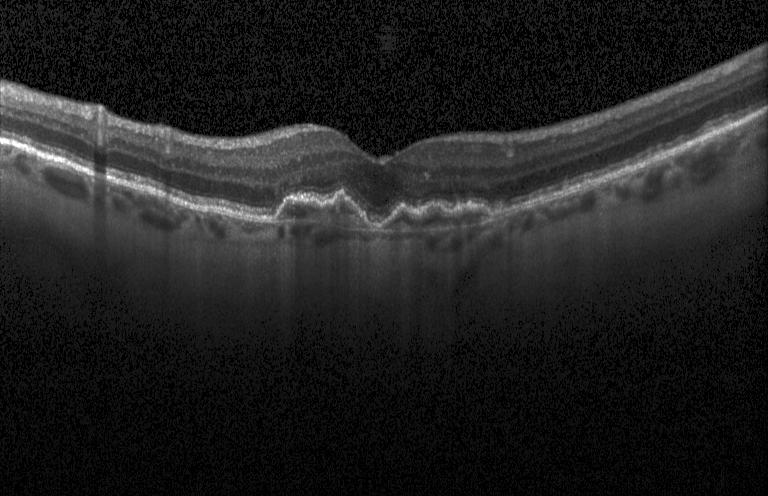 Macular scan. Optical coherence tomography scan. SD-OCT — This B-scan demonstrates choroidal neovascularization (CNV).